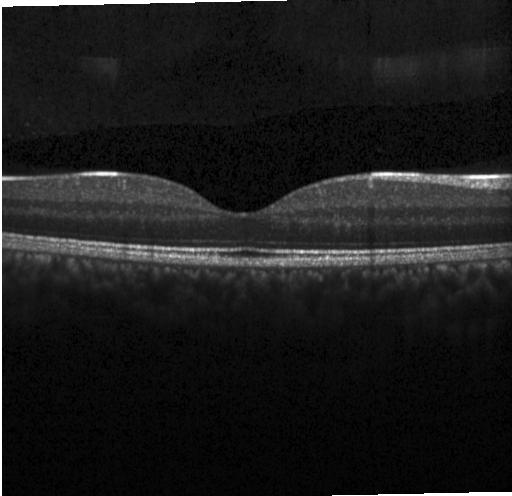
Assessment: no evidence of choroidal neovascularization, diabetic macular edema, or drusen.